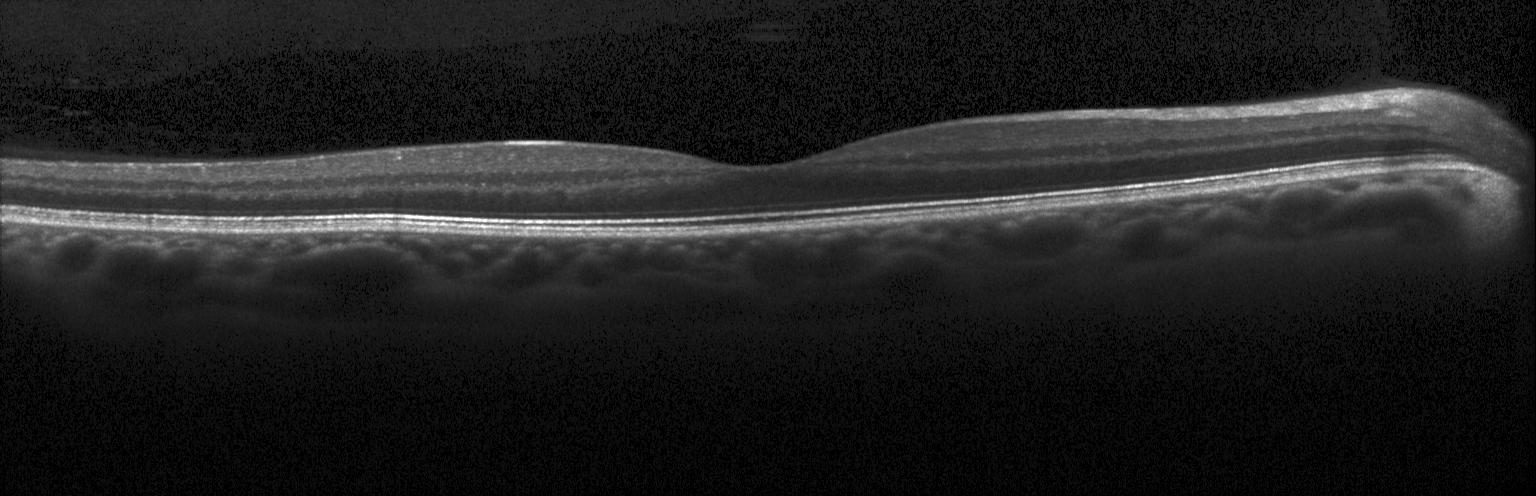
OCT B-scan. Finding: neither CNV, DME, nor drusen.